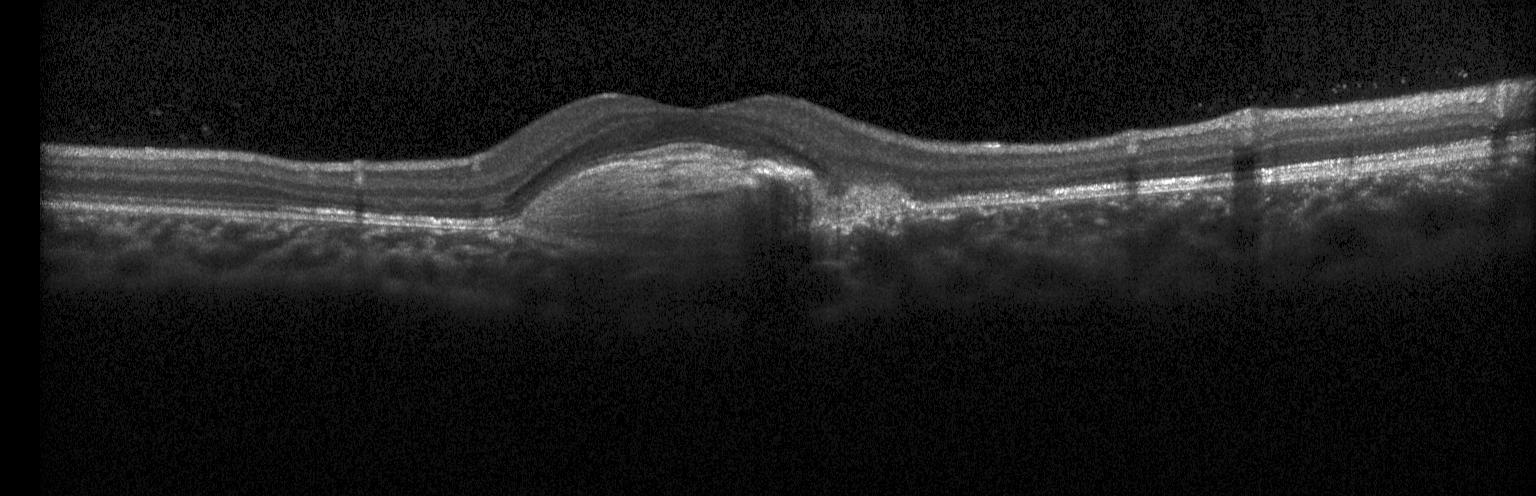 Spectral-domain OCT B-scan: a choroidal neovascular membrane.